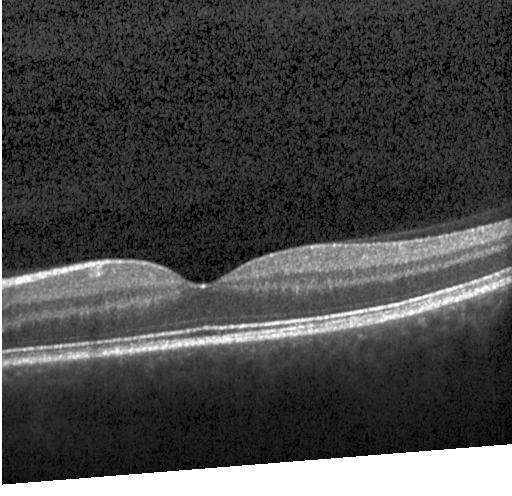 Retinal OCT cross-section · spectral-domain optical coherence tomography · centered on the fovea · Heidelberg Spectralis OCT system
Dx: no CNV, no DME, and no drusen.